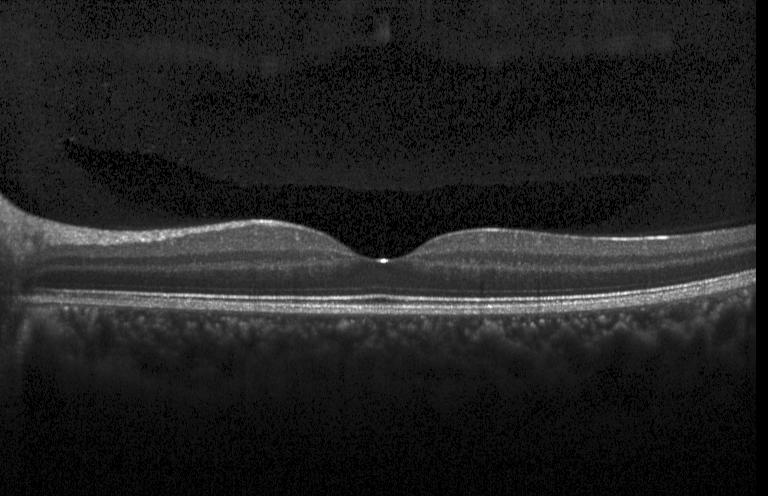
Spectral-domain optical coherence tomography. Fovea-centered. Retinal OCT B-scan. Heidelberg Spectralis OCT system. This B-scan demonstrates neither choroidal neovascularization, diabetic macular edema, nor drusen.